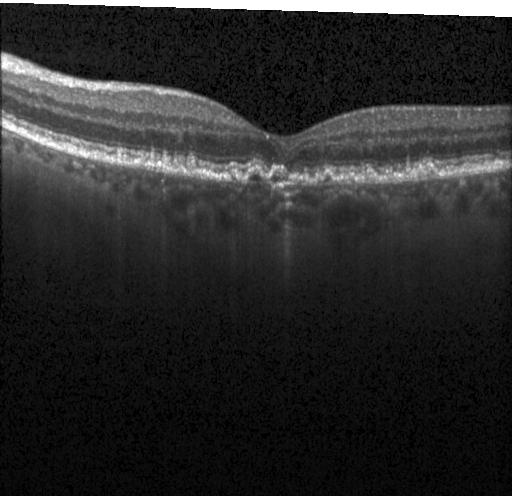
Spectral-domain OCT B-scan: a choroidal neovascular membrane.